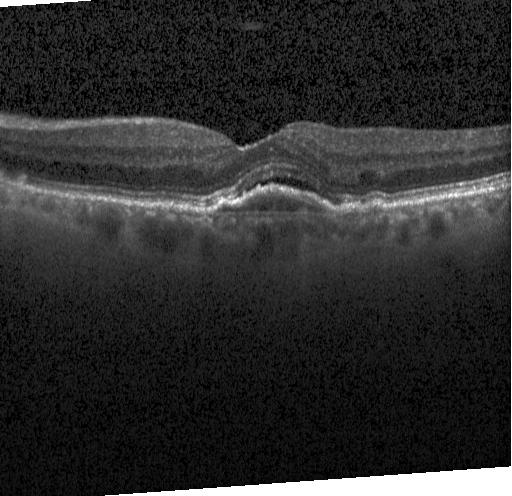

Acquired on a Heidelberg Spectralis; macular scan; optical coherence tomography B-scan.
Diagnosis: choroidal neovascularization (CNV).